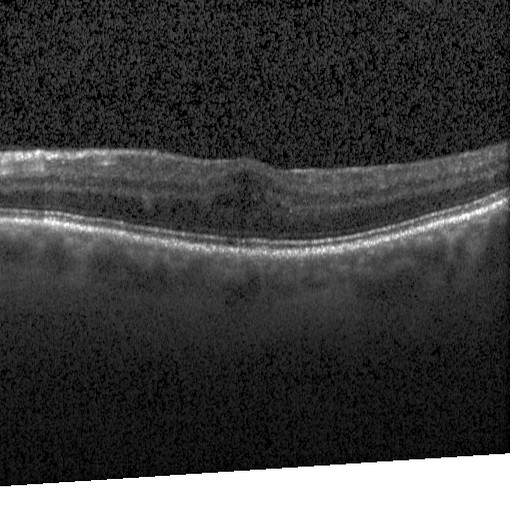
Macular scan. SD-OCT. Heidelberg Spectralis OCT system. Retinal OCT B-scan
Impression: diabetic macular edema.